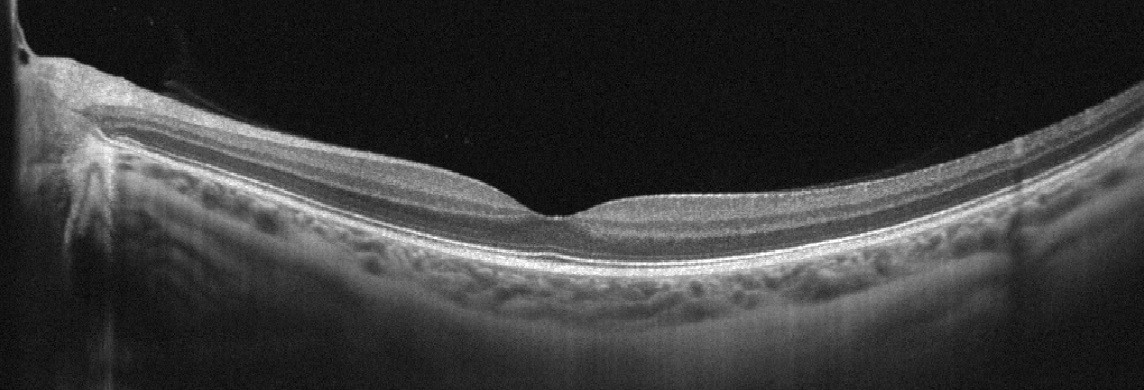

Acquired on an Optovue Avanti RTVue XR. Macular scan. Retinal OCT cross-section.
Diagnosis: no AMD, DME, ERM, RAO, RVO, or VID.